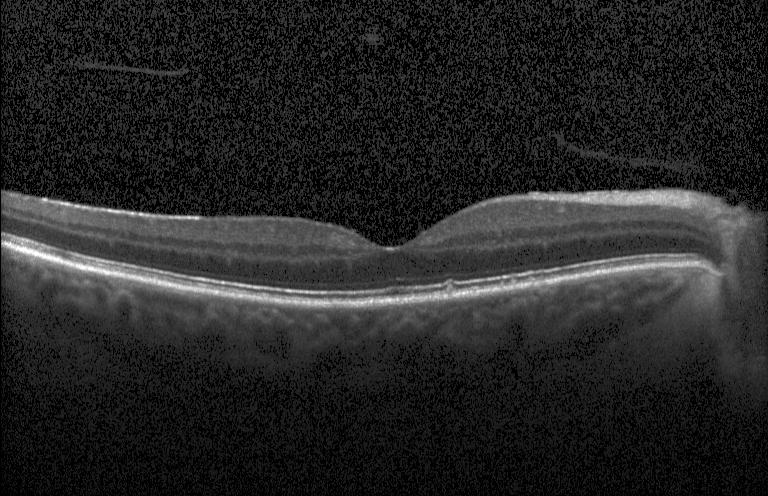

Optical coherence tomography B-scan — No evidence of CNV, DME, or drusen.